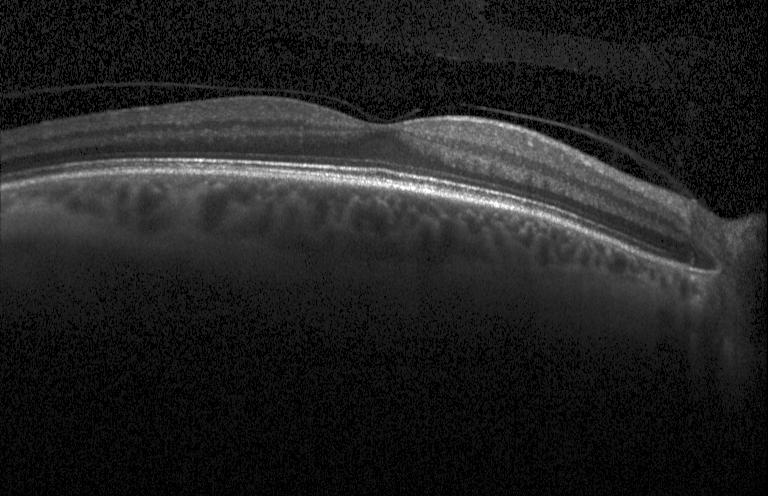 OCT B-scan, SD-OCT, centered on the fovea, acquired on a Heidelberg Spectralis. Impression: no choroidal neovascularization, diabetic macular edema, or drusen.